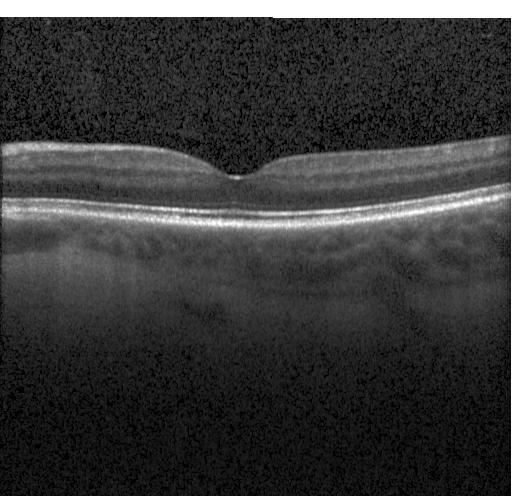

Retinal OCT cross-section showing neither CNV, DME, nor drusen.